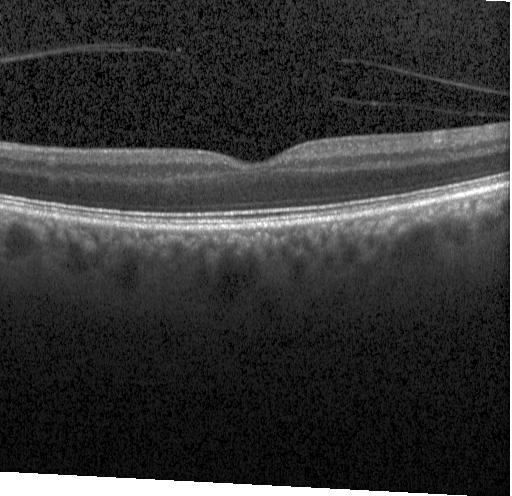 Heidelberg Spectralis · fovea-centered · retinal OCT cross-section · spectral-domain optical coherence tomography
Finding: no evidence of choroidal neovascularization, diabetic macular edema, or drusen.